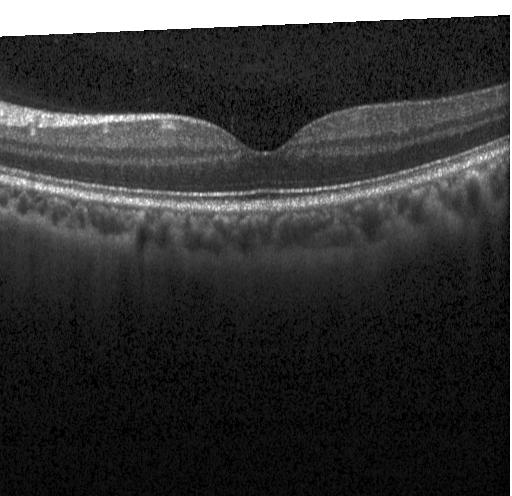
Optical coherence tomography scan, spectral-domain optical coherence tomography, acquired on a Heidelberg Spectralis, through the macula
This B-scan demonstrates neither CNV, DME, nor drusen.